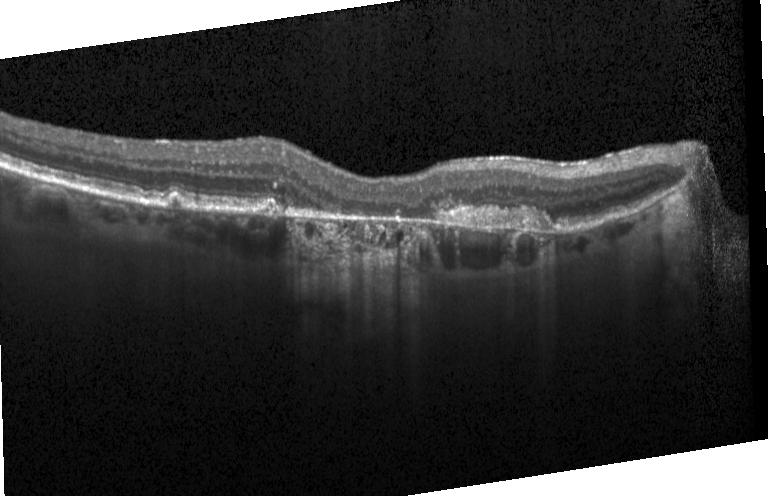 Macular OCT: a choroidal neovascular membrane.